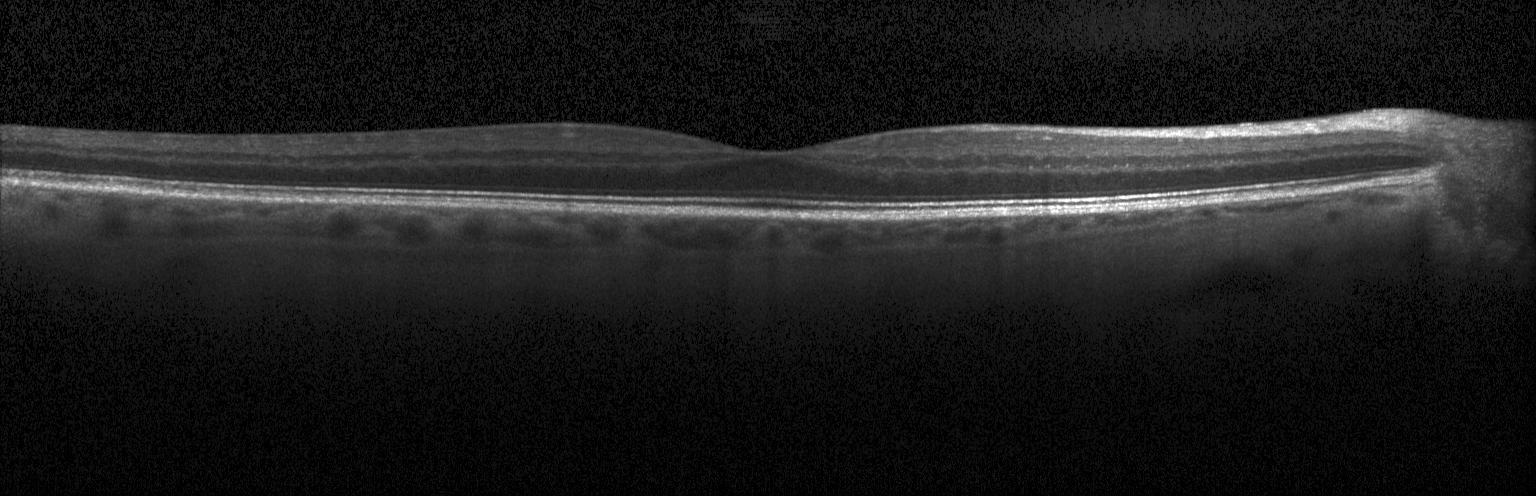

OCT B-scan · Heidelberg Spectralis · fovea-centered.
Finding: neither CNV, DME, nor drusen.